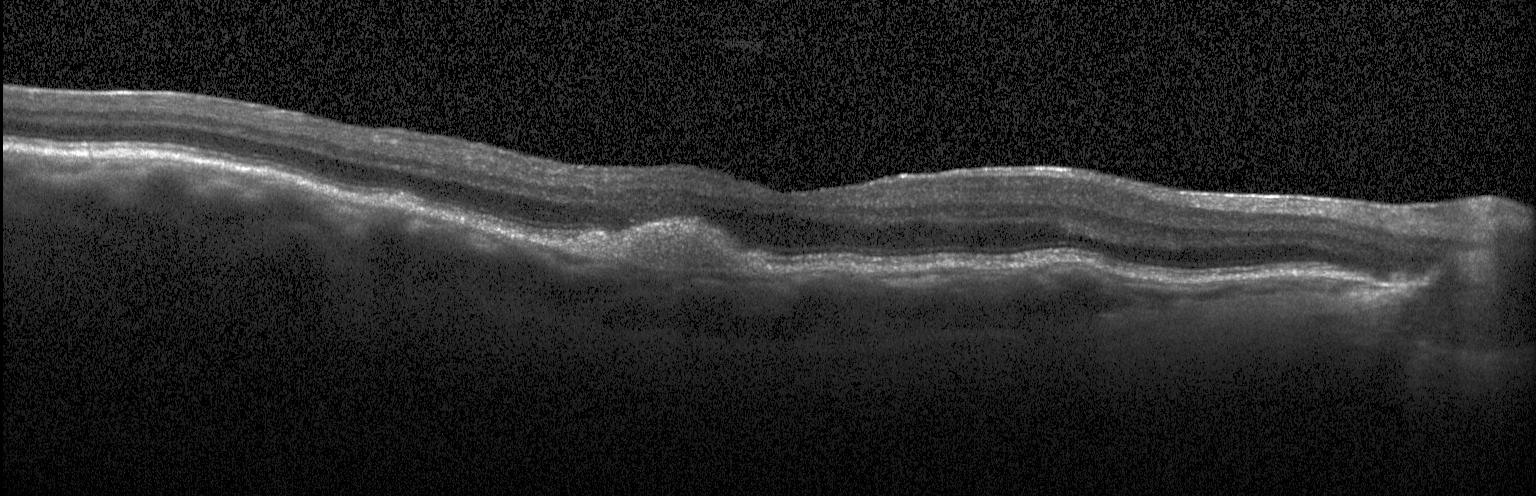

This B-scan demonstrates choroidal neovascularization (CNV).